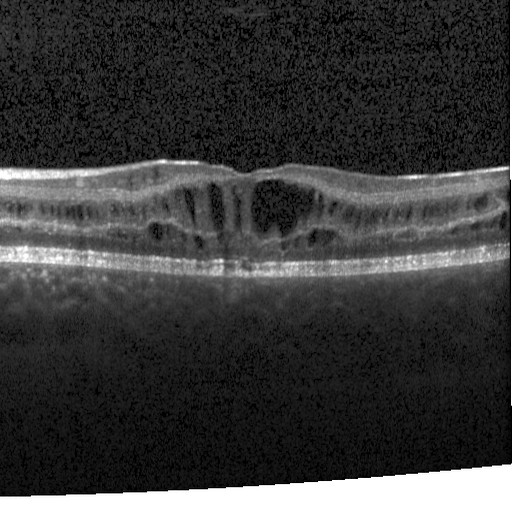

OCT B-scan; macular scan. Diagnosis: diabetic macular edema (DME).